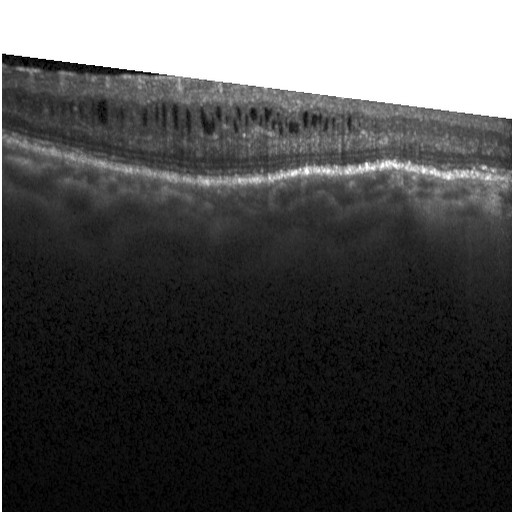 OCT finding: diabetic macular edema.